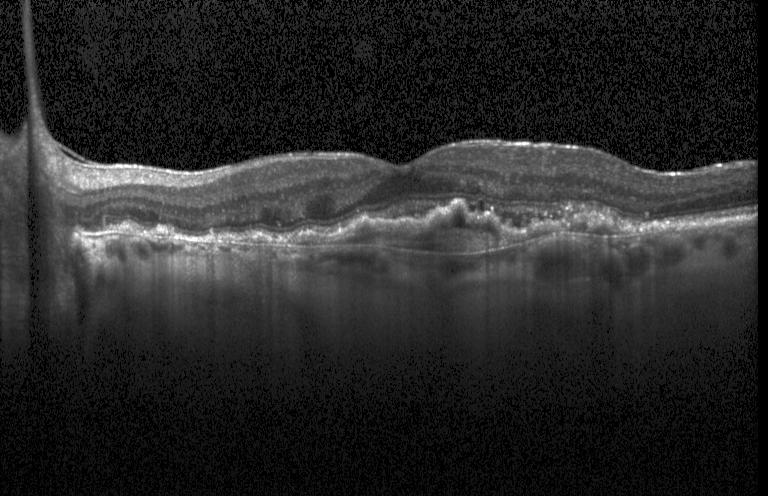 Acquired on a Heidelberg Spectralis; optical coherence tomography B-scan.
Impression: a choroidal neovascular membrane.